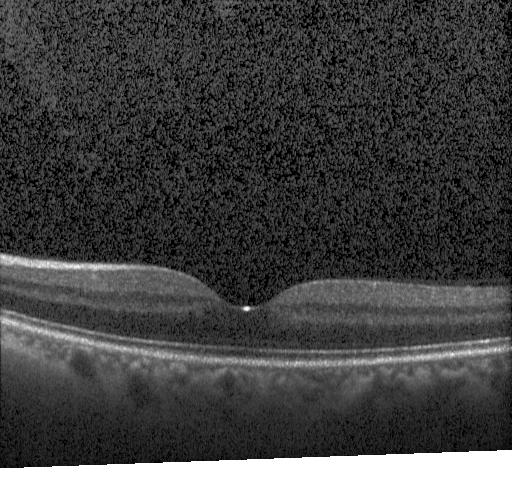
Fovea-centered; acquired on a Heidelberg Spectralis; spectral-domain OCT; retinal OCT B-scan. Impression: no CNV, DME, or drusen.